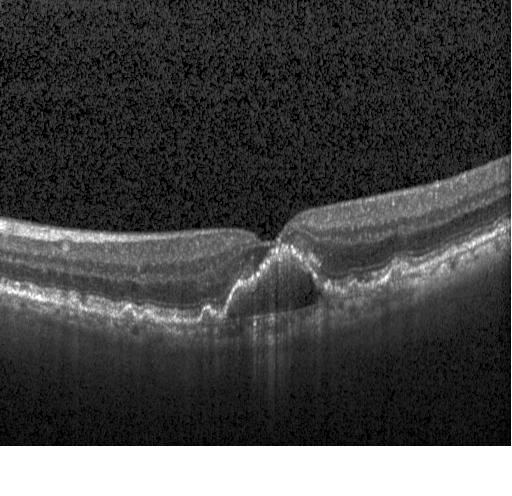
Optical coherence tomography scan — Finding: choroidal neovascularization (CNV).